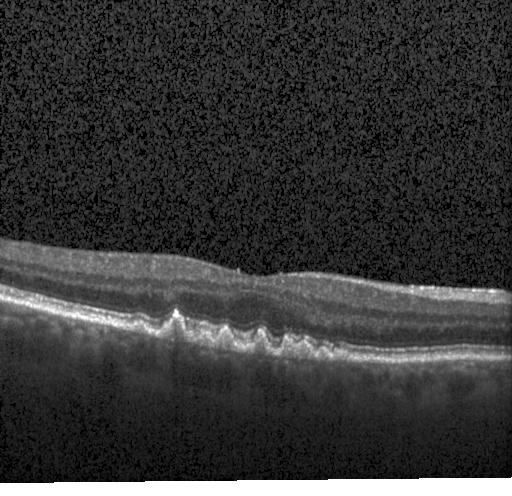

Finding: sub-RPE drusenoid deposits.